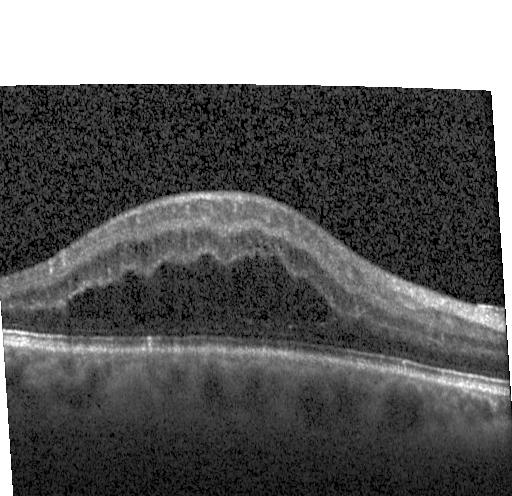

Retinal OCT B-scan.
The scan shows DME.